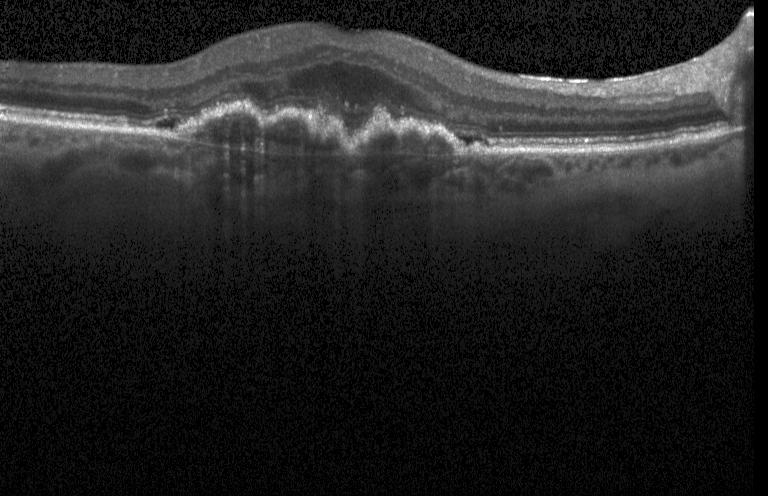 The scan shows choroidal neovascularization.